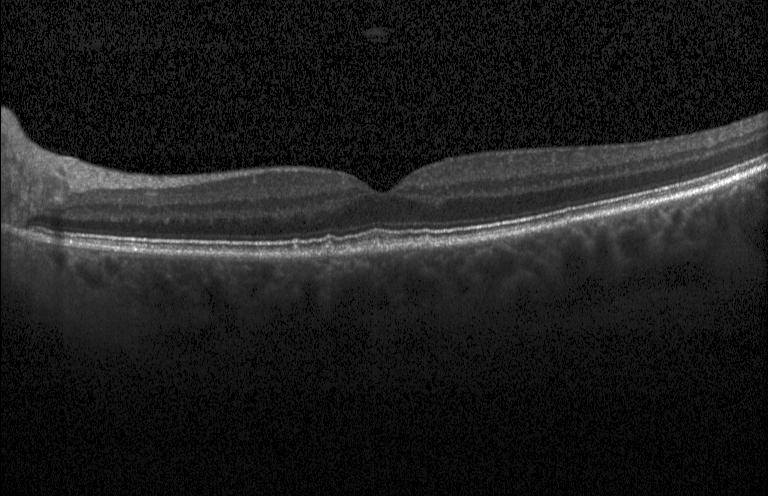
Impression: drusen.